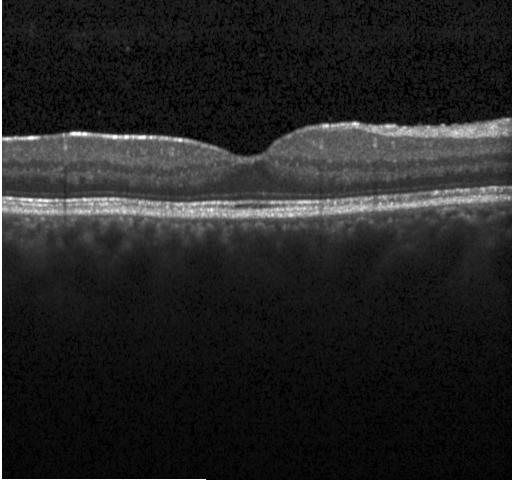
Spectral-domain OCT, retinal OCT B-scan
Dx: no choroidal neovascularization, diabetic macular edema, or drusen.